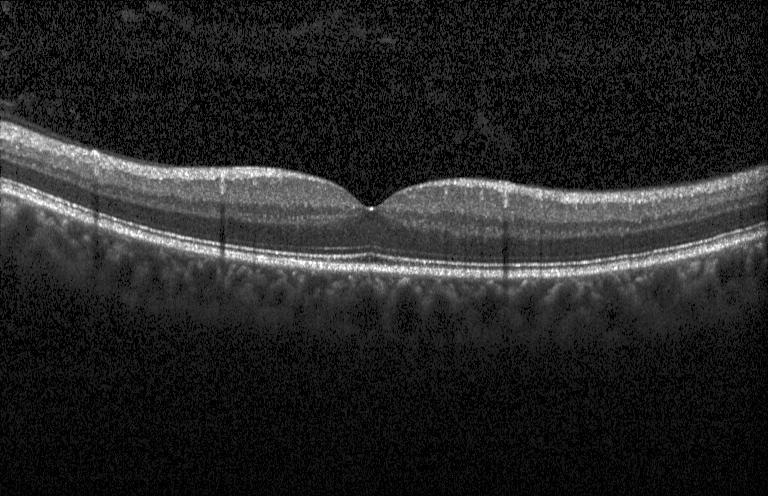

Assessment: no CNV, DME, or drusen.